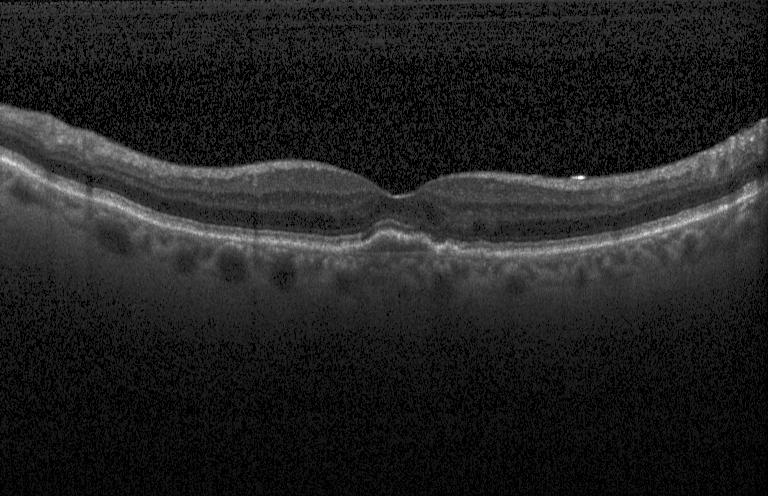 Finding: a choroidal neovascular membrane.